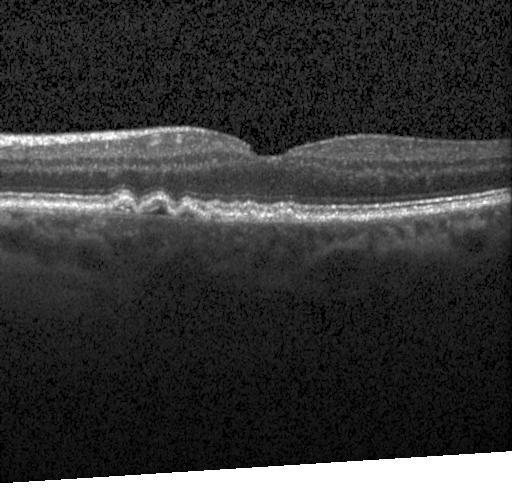
OCT B-scan. Diagnosis: multiple drusen.